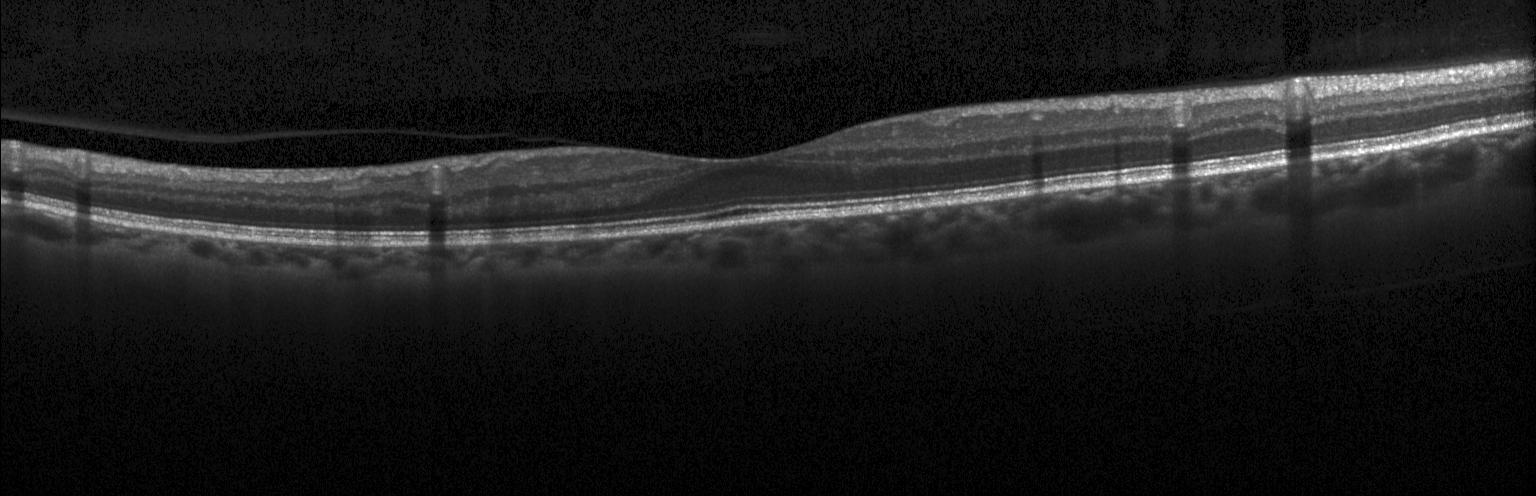 Impression: no evidence of choroidal neovascularization, diabetic macular edema, or drusen.